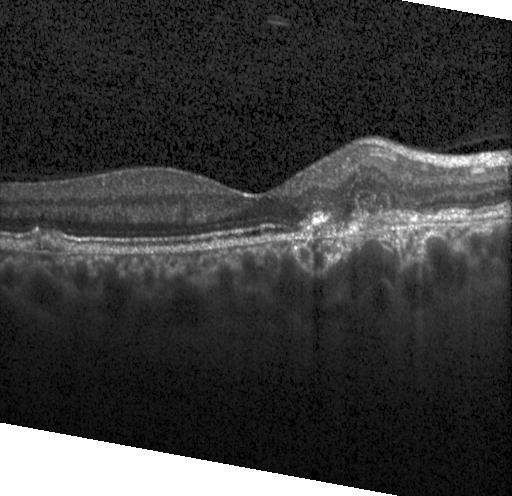
Optical coherence tomography B-scan; spectral-domain optical coherence tomography; through the macula; Heidelberg Spectralis OCT system — CNV.